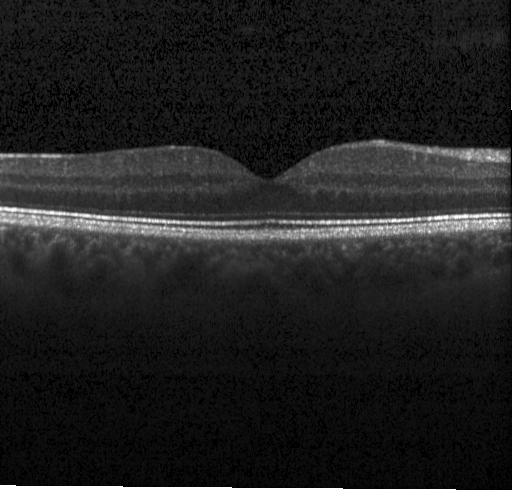
Spectral-domain OCT · retinal OCT cross-section · Heidelberg Spectralis OCT system — Assessment: neither CNV, DME, nor drusen.